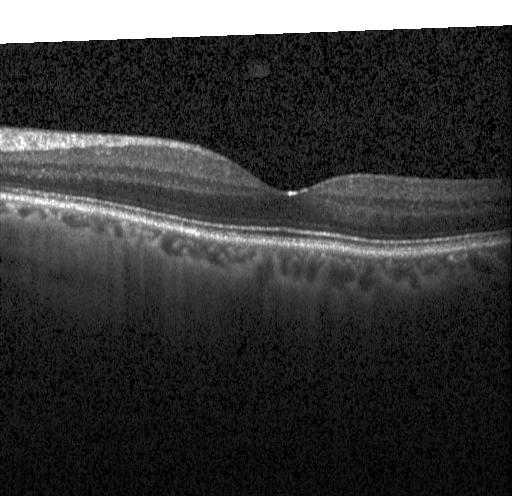 Optical coherence tomography B-scan · acquired on a Heidelberg Spectralis.
OCT finding: no CNV, DME, or drusen.